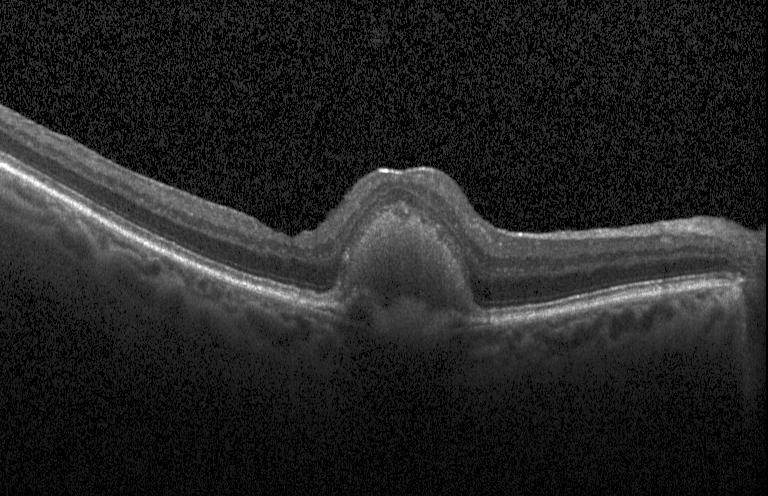 This B-scan demonstrates CNV.